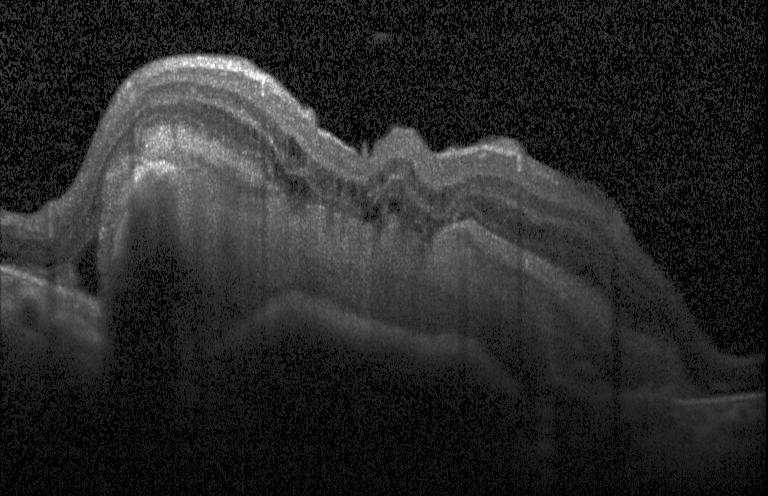

Diagnosis: choroidal neovascularization.